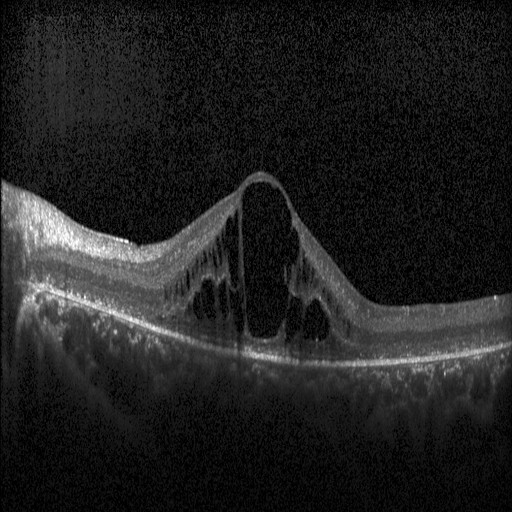 Diagnosis: diabetic macular edema (DME).